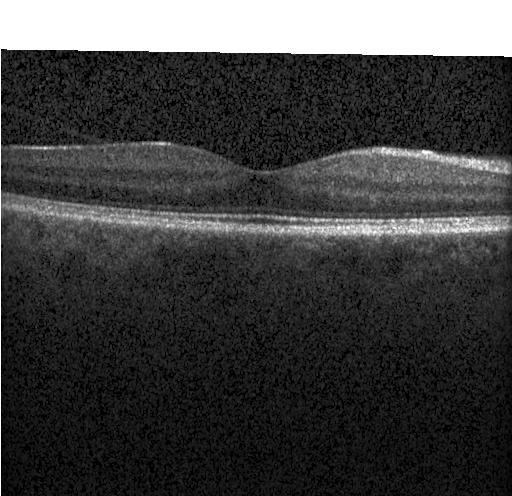

Optical coherence tomography scan; SD-OCT; centered on the fovea. Impression: no choroidal neovascularization, diabetic macular edema, or drusen.